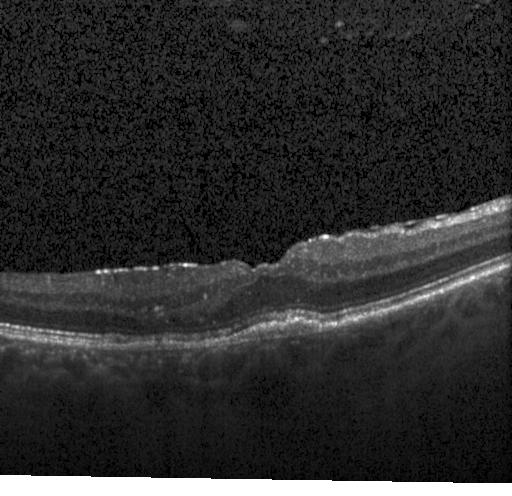 OCT line scan
Assessment: a choroidal neovascular membrane.